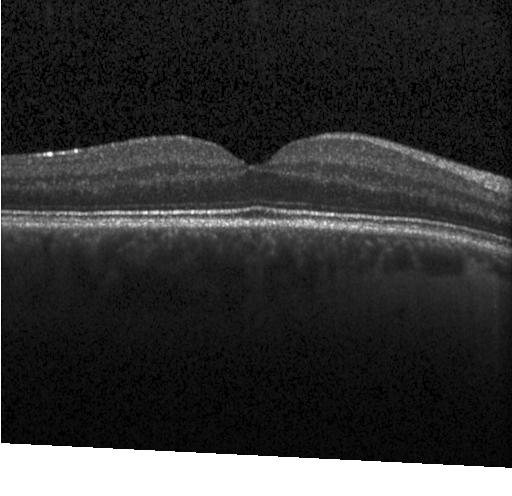

Finding: no evidence of CNV, DME, or drusen.